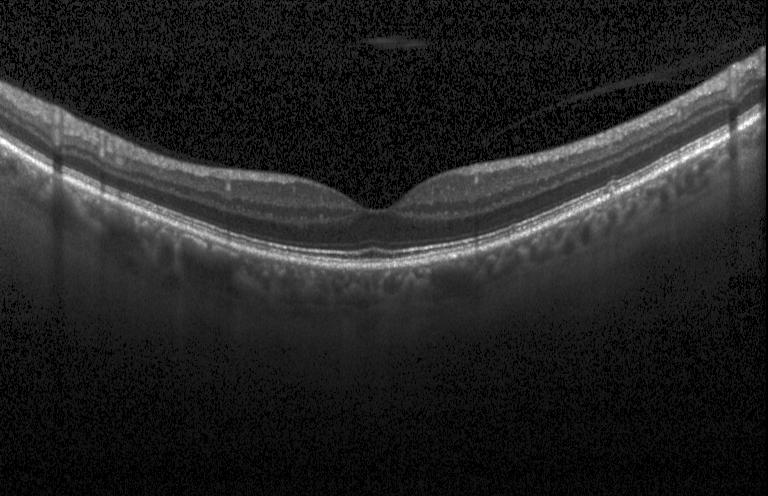 Retinal OCT B-scan.
Assessment: no evidence of choroidal neovascularization, diabetic macular edema, or drusen.